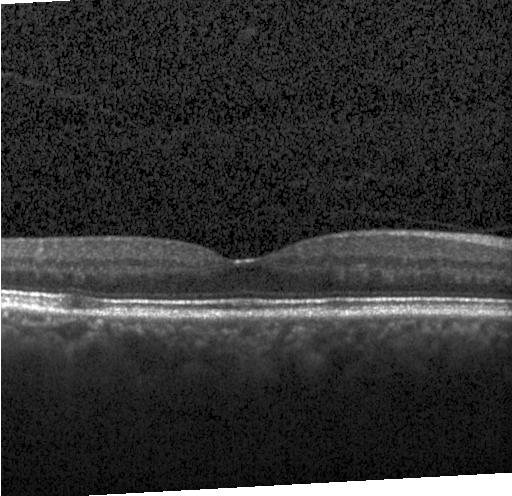
Acquired on a Heidelberg Spectralis · through the macula · optical coherence tomography B-scan · spectral-domain optical coherence tomography
Finding: neither choroidal neovascularization, diabetic macular edema, nor drusen.